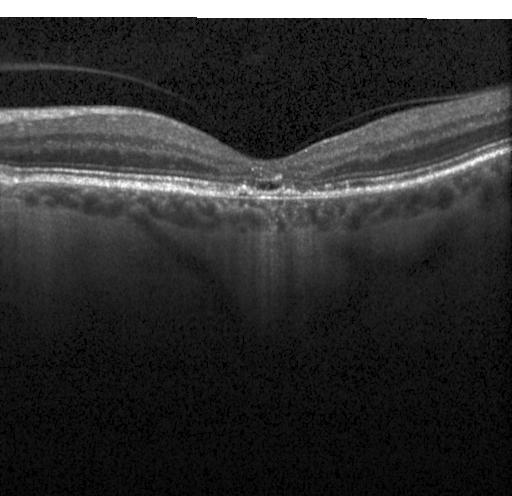
OCT B-scan. Diagnosis: CNV.